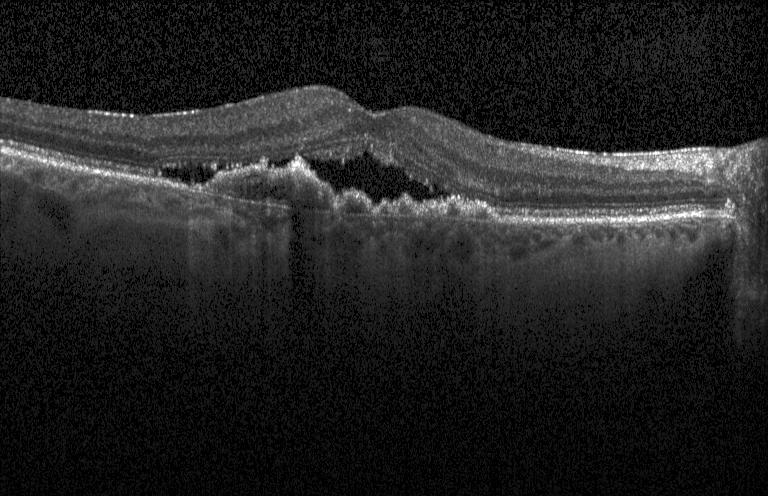
This B-scan demonstrates CNV.